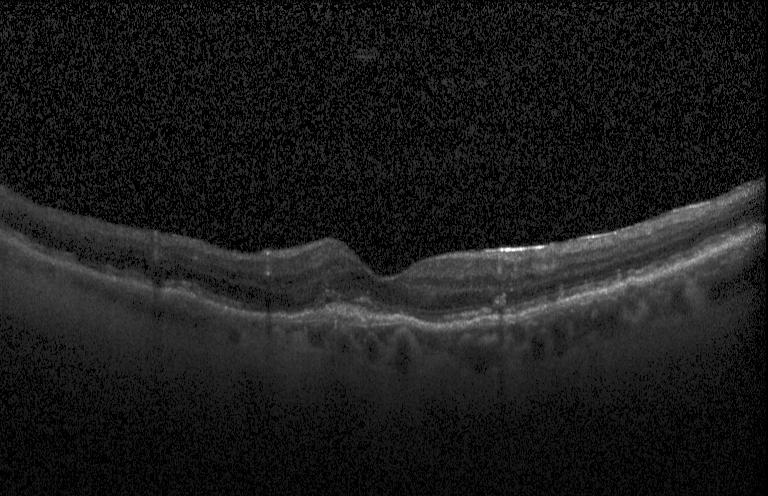

OCT B-scan. Diagnosis: choroidal neovascularization (CNV).